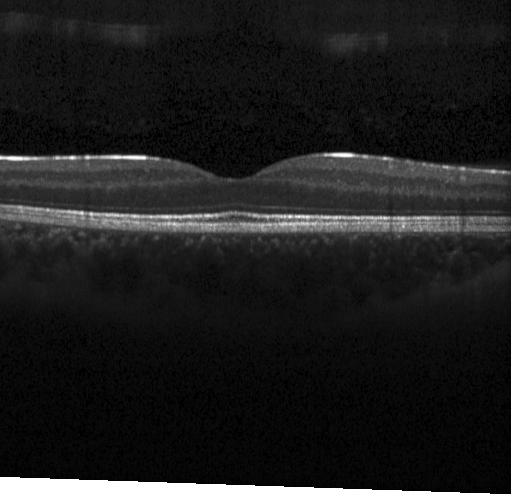
Acquired on a Heidelberg Spectralis, through the macula, OCT line scan — Finding: no evidence of choroidal neovascularization, diabetic macular edema, or drusen.